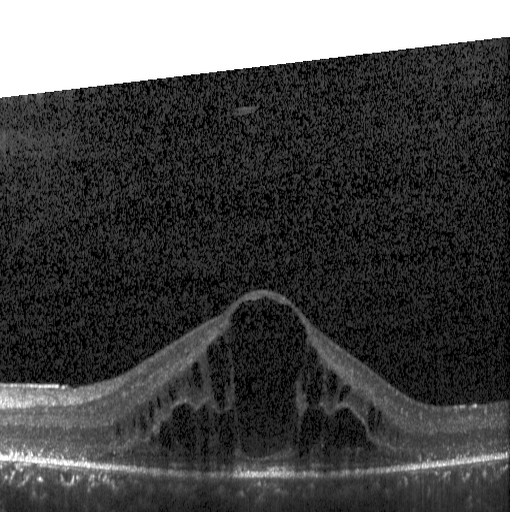 OCT B-scan.
OCT finding: diabetic macular edema (DME).